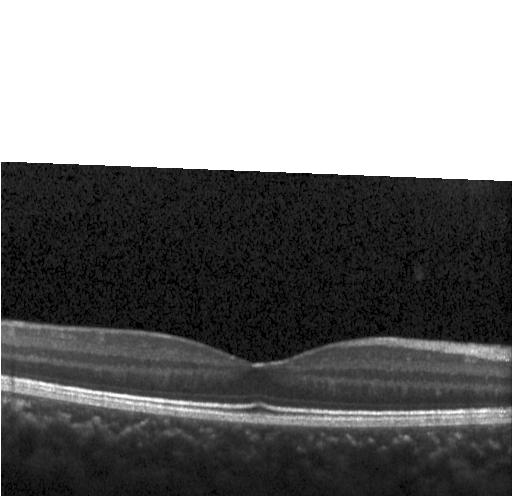

Spectral-domain optical coherence tomography; retinal OCT B-scan; acquired on a Heidelberg Spectralis; fovea-centered.
Finding: neither choroidal neovascularization, diabetic macular edema, nor drusen.